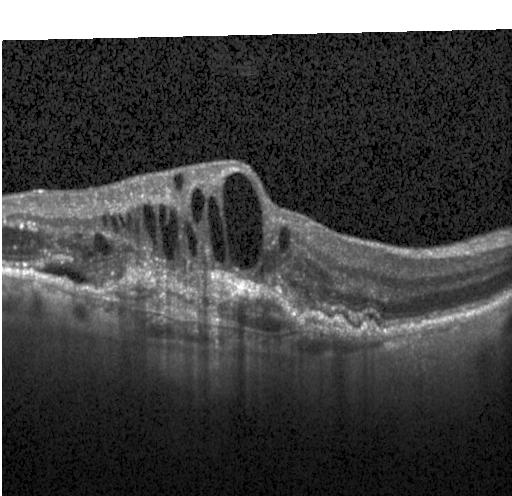

Retinal OCT cross-section.
Impression: CNV.